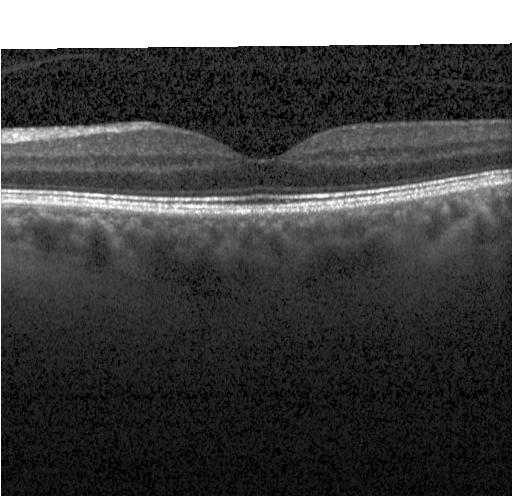

Diagnosis: no choroidal neovascularization, no diabetic macular edema, and no drusen.